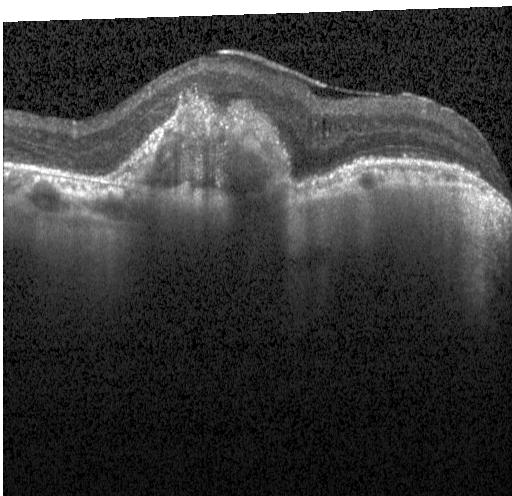

Spectral-domain OCT; optical coherence tomography B-scan; acquired on a Heidelberg Spectralis — Macular OCT: a choroidal neovascular membrane.